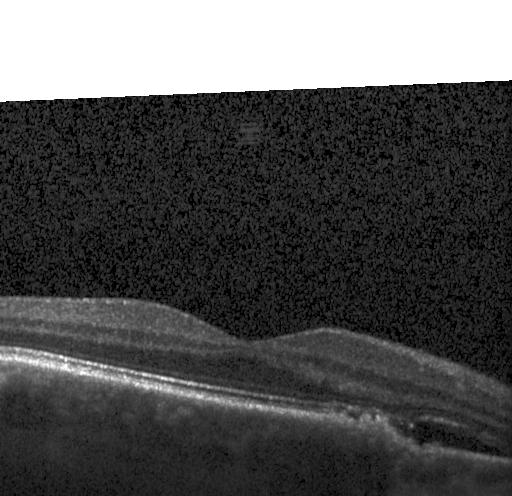

Diagnosis: a choroidal neovascular membrane.